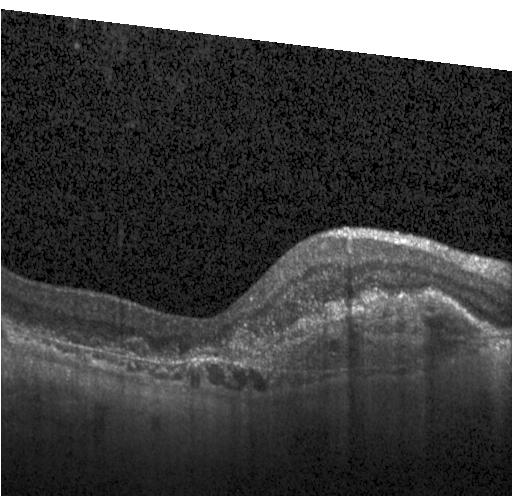

Heidelberg Spectralis OCT system; optical coherence tomography B-scan; horizontal scan through the fovea. Impression: CNV.